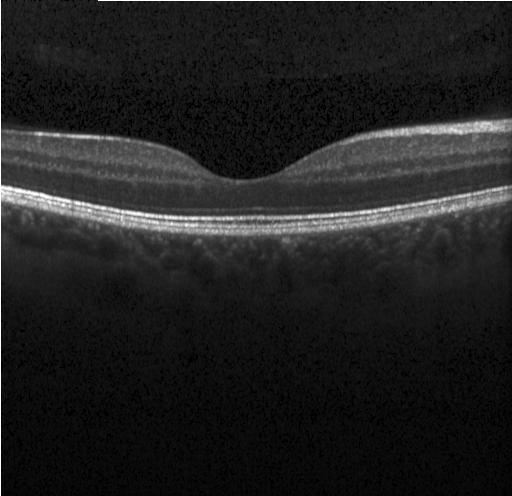

Optical coherence tomography scan. Diagnosis: no choroidal neovascularization, diabetic macular edema, or drusen.